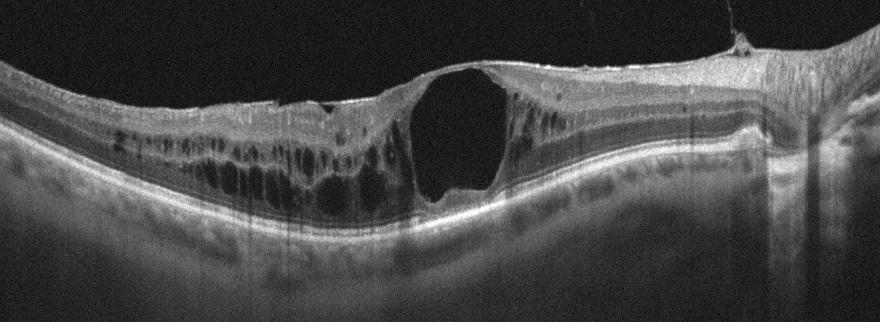

OCT B-scan showing diabetic macular edema (DME).